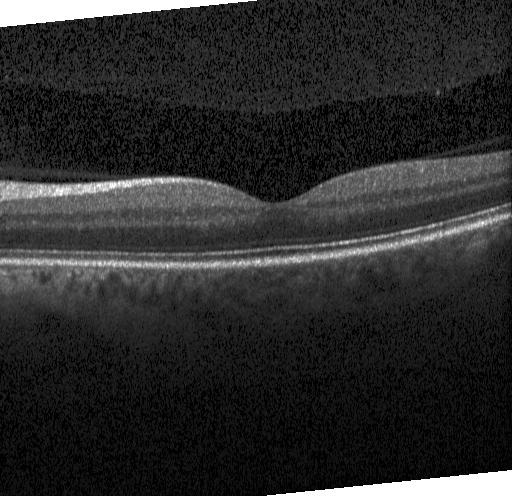

Optical coherence tomography scan · SD-OCT · instrument: Heidelberg Spectralis.
OCT finding: no evidence of choroidal neovascularization, diabetic macular edema, or drusen.